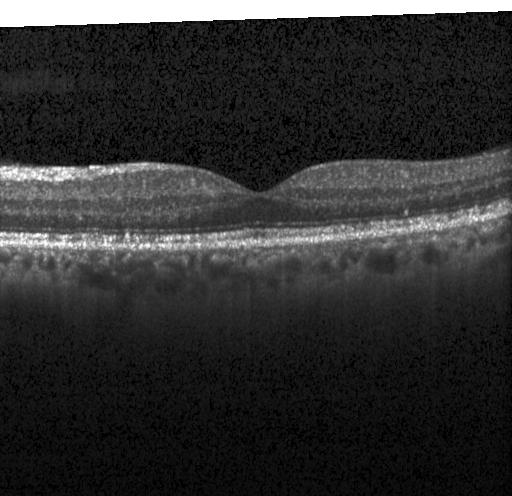 Spectral-domain optical coherence tomography · instrument: Heidelberg Spectralis · macular scan · optical coherence tomography scan.
OCT finding: neither choroidal neovascularization, diabetic macular edema, nor drusen.